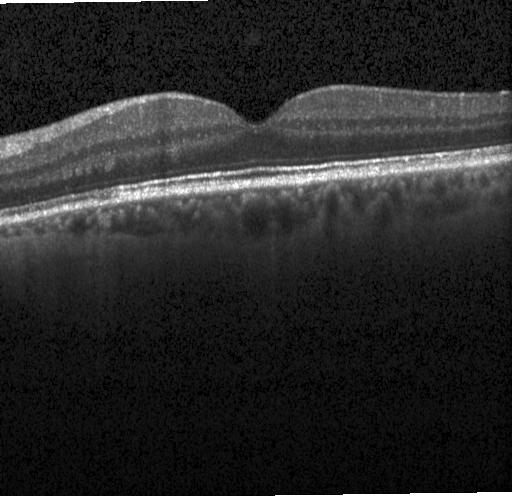

Instrument: Heidelberg Spectralis · retinal OCT cross-section · macular scan · spectral-domain optical coherence tomography. Impression: no choroidal neovascularization, no diabetic macular edema, and no drusen.